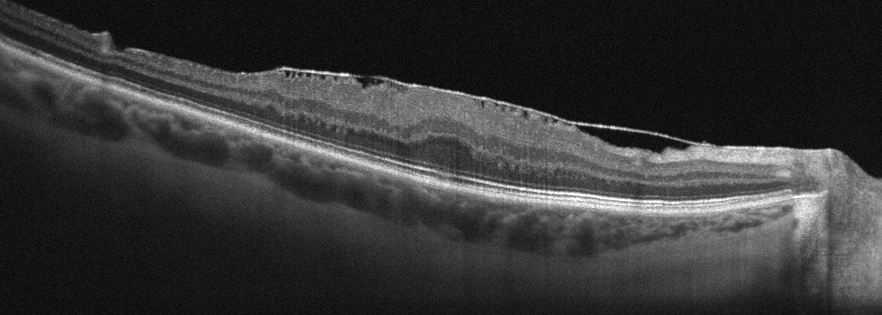
Left eye · OCT B-scan. Diagnosis: ERM.